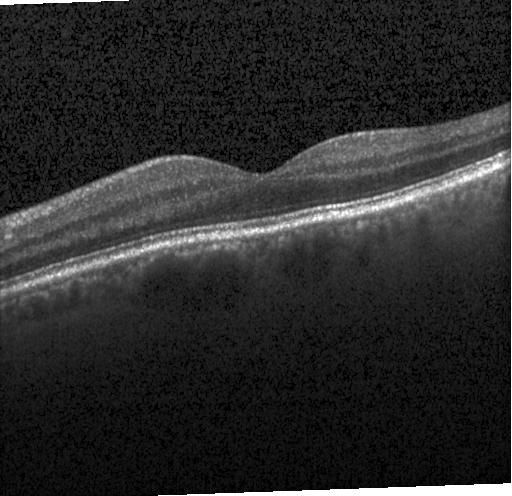 Through the macula; Heidelberg Spectralis; optical coherence tomography B-scan. Diagnosis: neither choroidal neovascularization, diabetic macular edema, nor drusen.